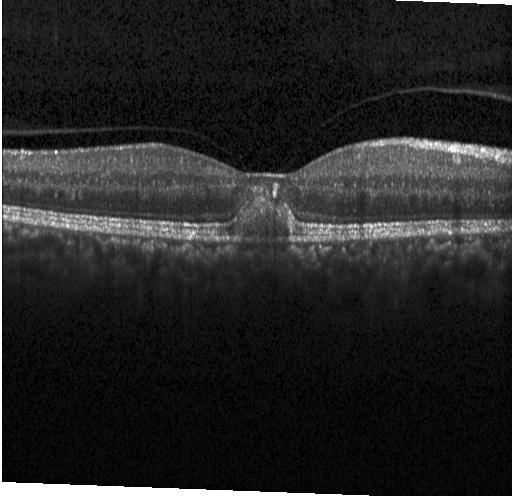
Optical coherence tomography B-scan. Heidelberg Spectralis OCT system. Fovea-centered. Spectral-domain optical coherence tomography — CNV.